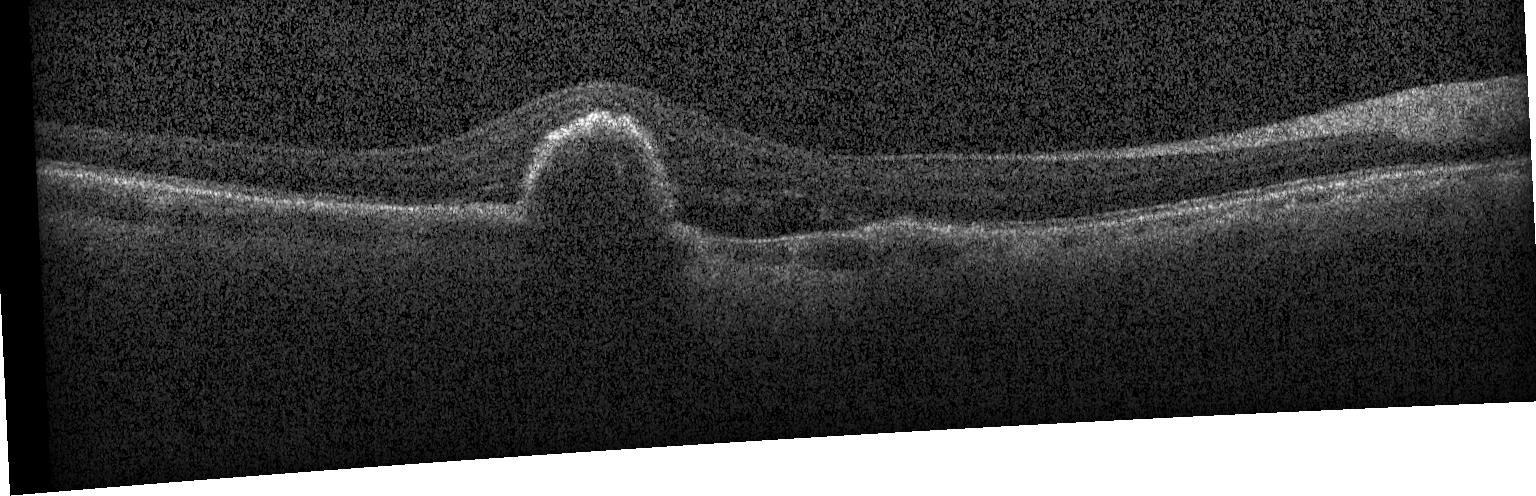 Spectral-domain OCT B-scan: choroidal neovascularization (CNV).